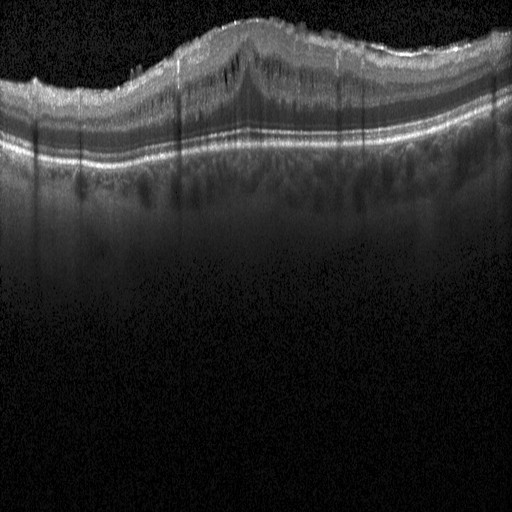
Macular OCT demonstrating diabetic macular edema (DME).